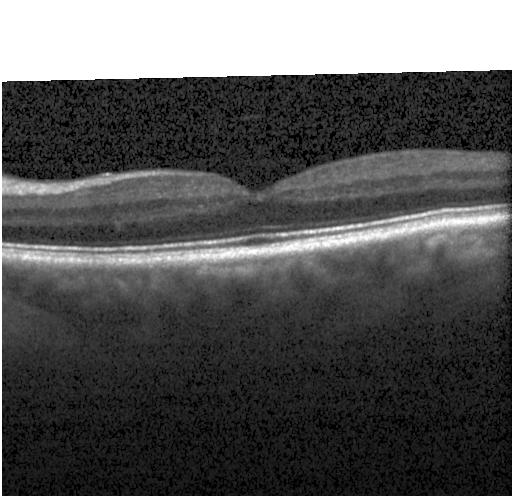
Heidelberg Spectralis · SD-OCT · through the macula · optical coherence tomography scan — This B-scan demonstrates neither CNV, DME, nor drusen.